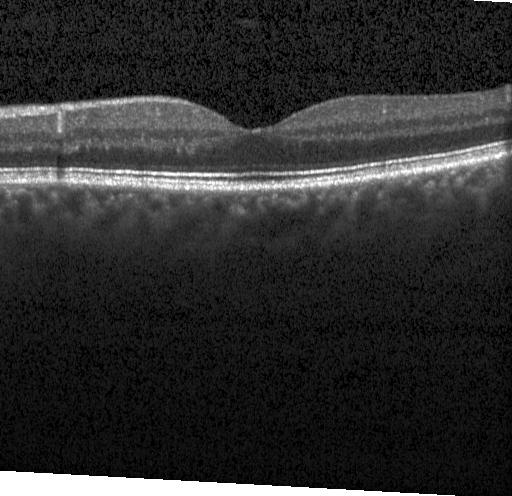
Heidelberg Spectralis OCT system, retinal OCT B-scan
The scan shows no choroidal neovascularization, diabetic macular edema, or drusen.